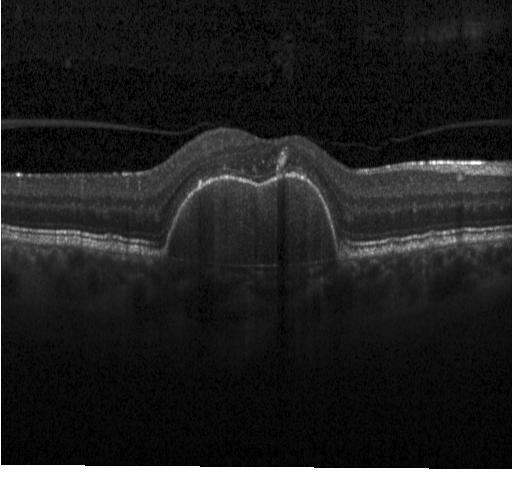 Macular scan. Optical coherence tomography scan
Impression: choroidal neovascularization (CNV).